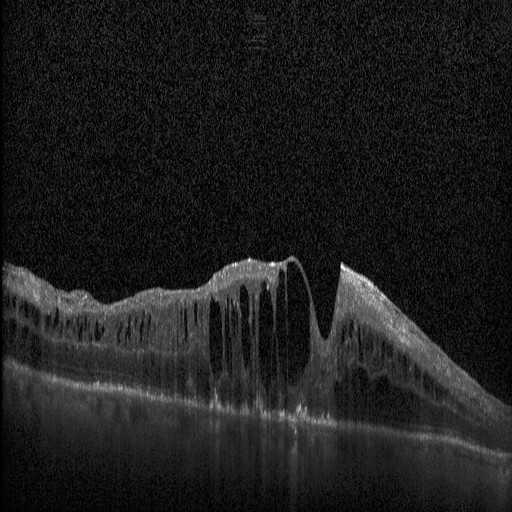 OCT B-scan showing diabetic macular edema.